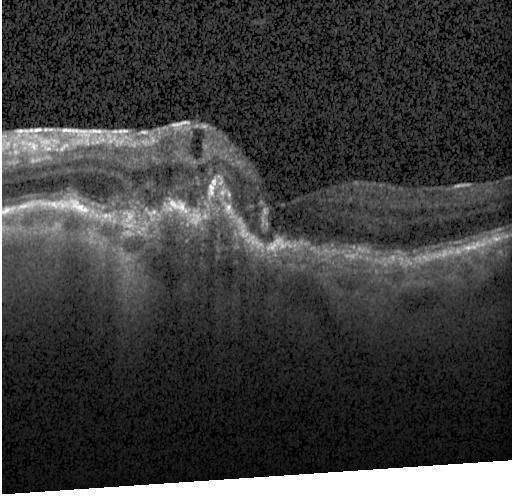 Optical coherence tomography B-scan; horizontal scan through the fovea
This B-scan demonstrates choroidal neovascularization (CNV).